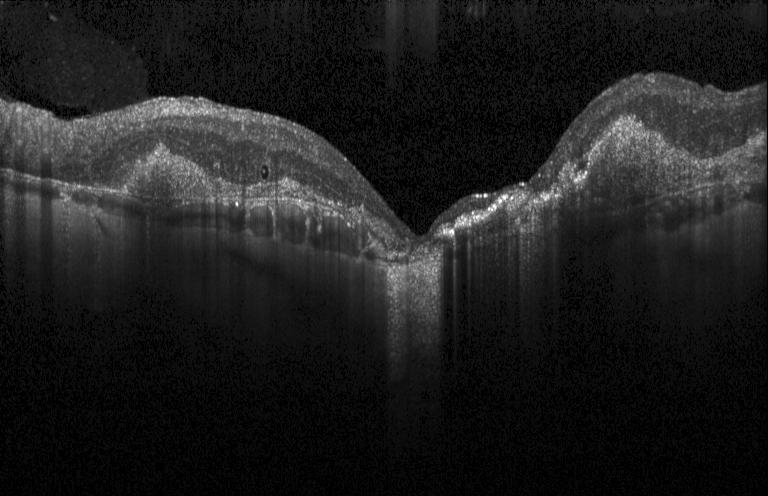

Finding: choroidal neovascularization.